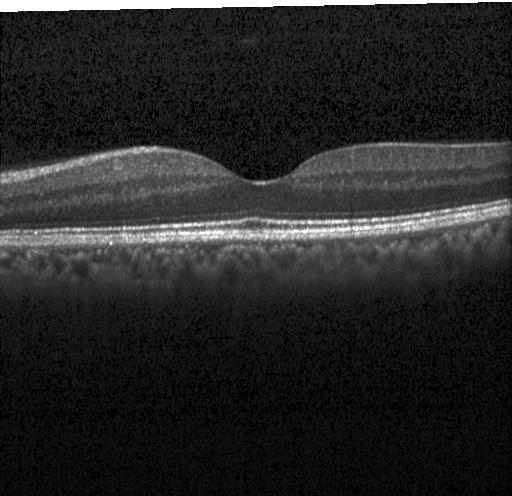
Spectral-domain OCT · acquired on a Heidelberg Spectralis · retinal OCT B-scan
Assessment: no evidence of choroidal neovascularization, diabetic macular edema, or drusen.